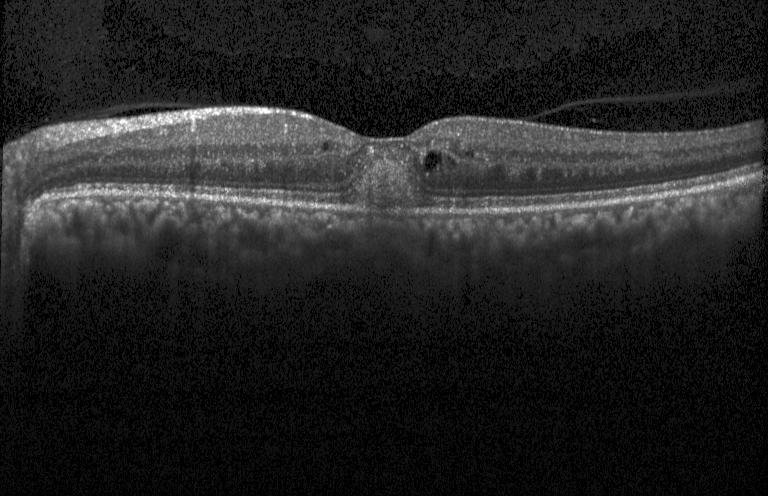

Diagnosis: a choroidal neovascular membrane.